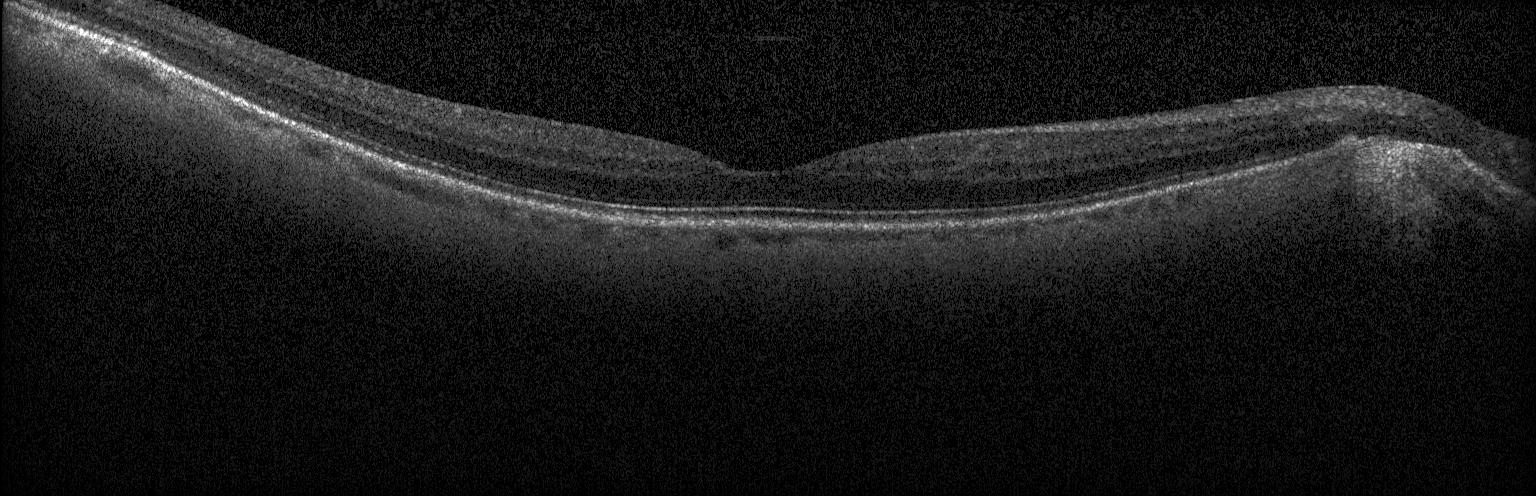 OCT scan showing neither choroidal neovascularization, diabetic macular edema, nor drusen.